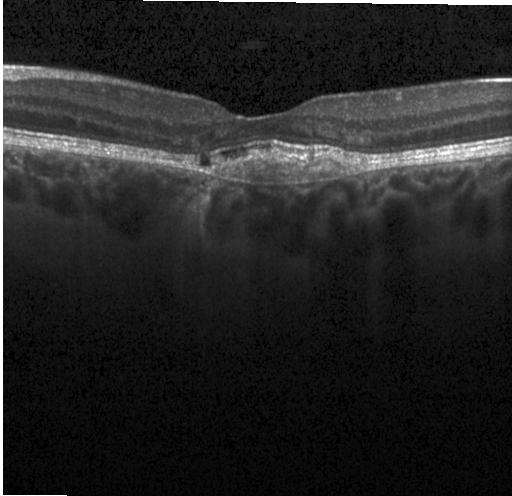
Instrument: Heidelberg Spectralis, centered on the fovea, optical coherence tomography B-scan, spectral-domain OCT. The scan shows a choroidal neovascular membrane.